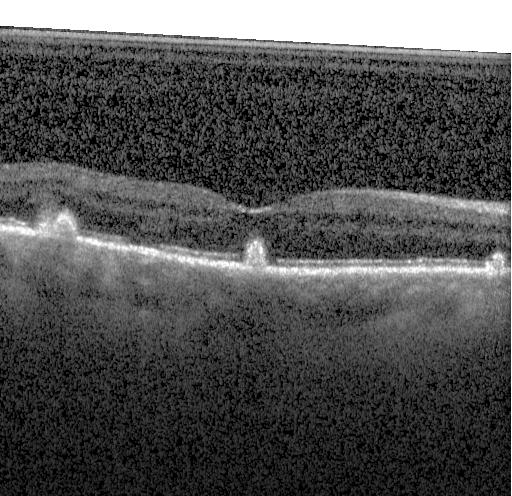 Optical coherence tomography B-scan
Macular OCT: multiple drusen.